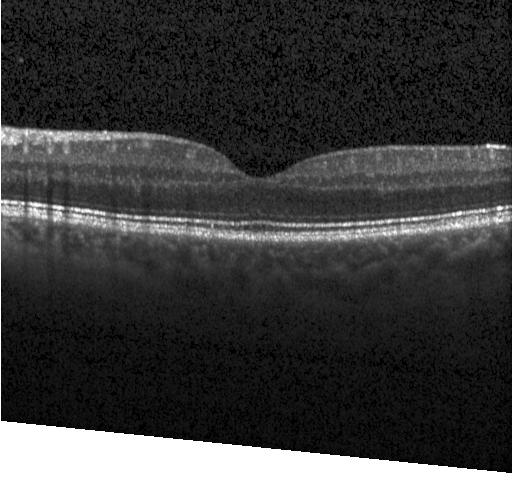 Fovea-centered · retinal OCT B-scan · spectral-domain OCT. Diagnosis: no evidence of choroidal neovascularization, diabetic macular edema, or drusen.